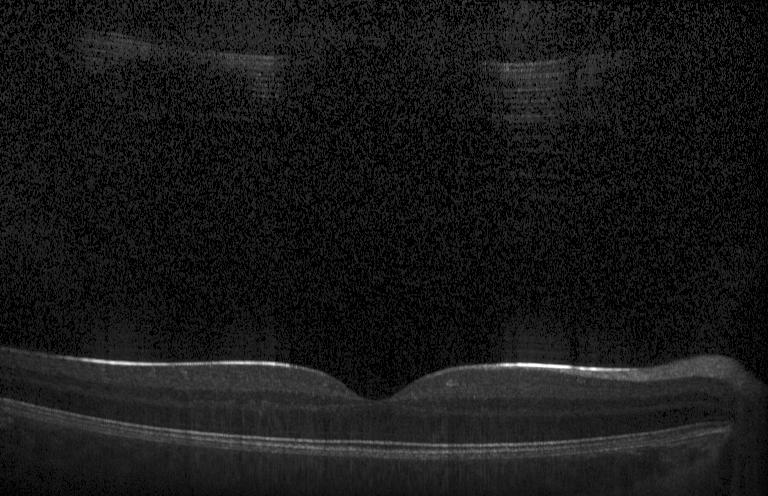 Acquired on a Heidelberg Spectralis. Macular scan. OCT B-scan — This B-scan demonstrates no choroidal neovascularization, diabetic macular edema, or drusen.